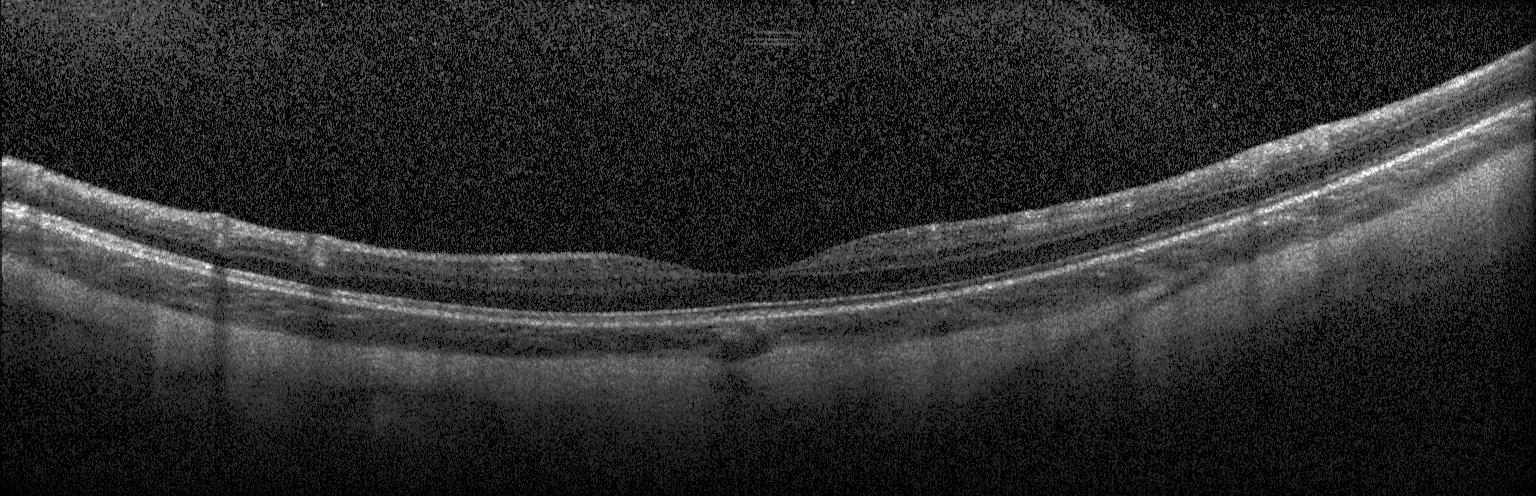
Optical coherence tomography scan; instrument: Heidelberg Spectralis
Finding: no evidence of choroidal neovascularization, diabetic macular edema, or drusen.